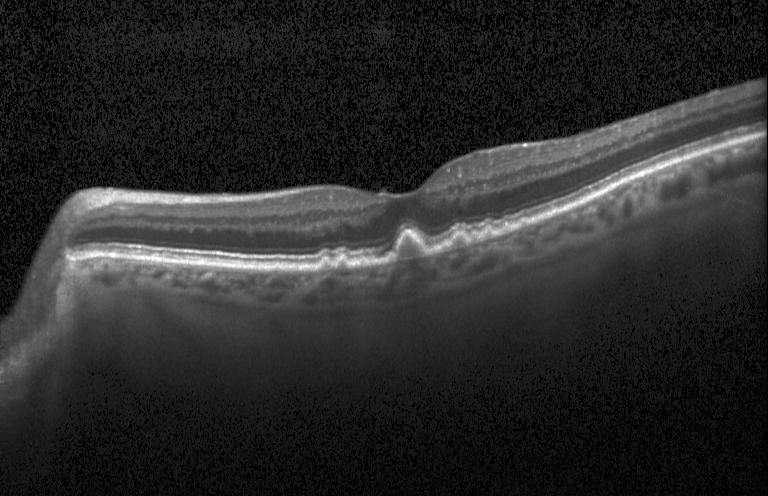 Dx: multiple drusen.